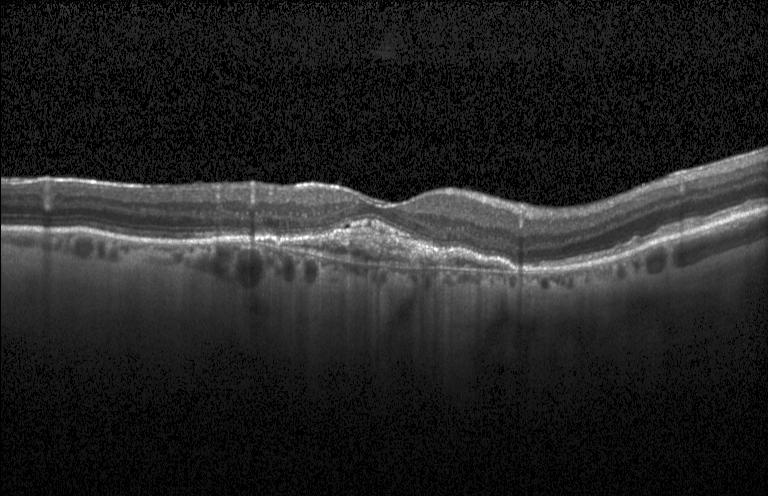
Optical coherence tomography B-scan. Spectral-domain optical coherence tomography. This B-scan demonstrates choroidal neovascularization (CNV).